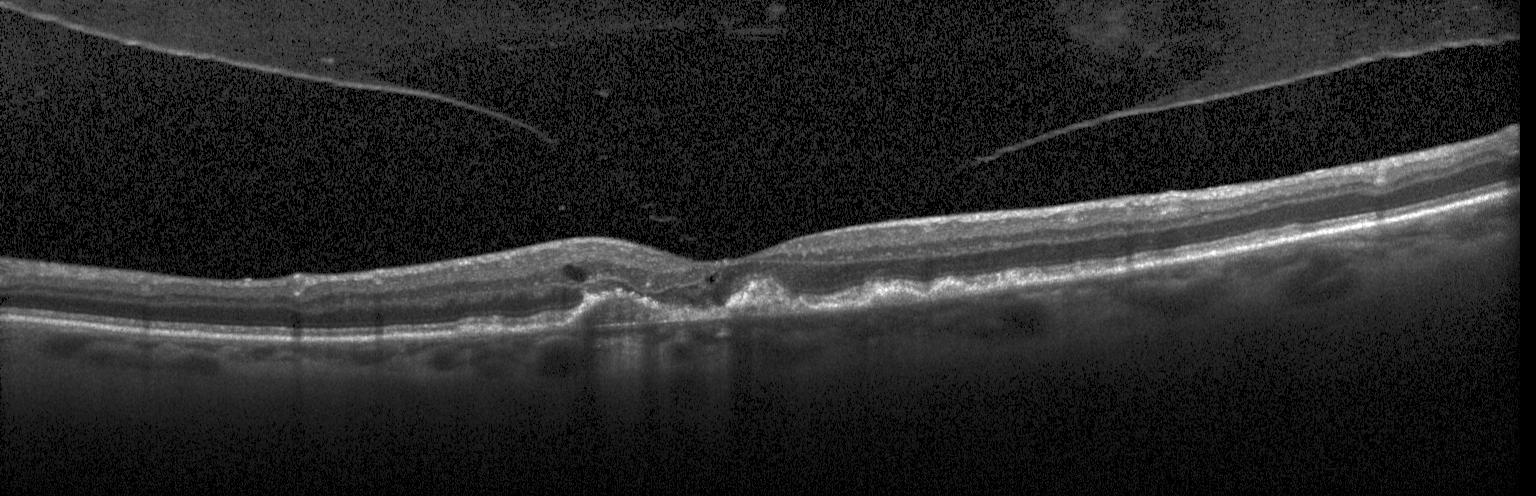
Acquired on a Heidelberg Spectralis, optical coherence tomography scan. Assessment: a choroidal neovascular membrane.